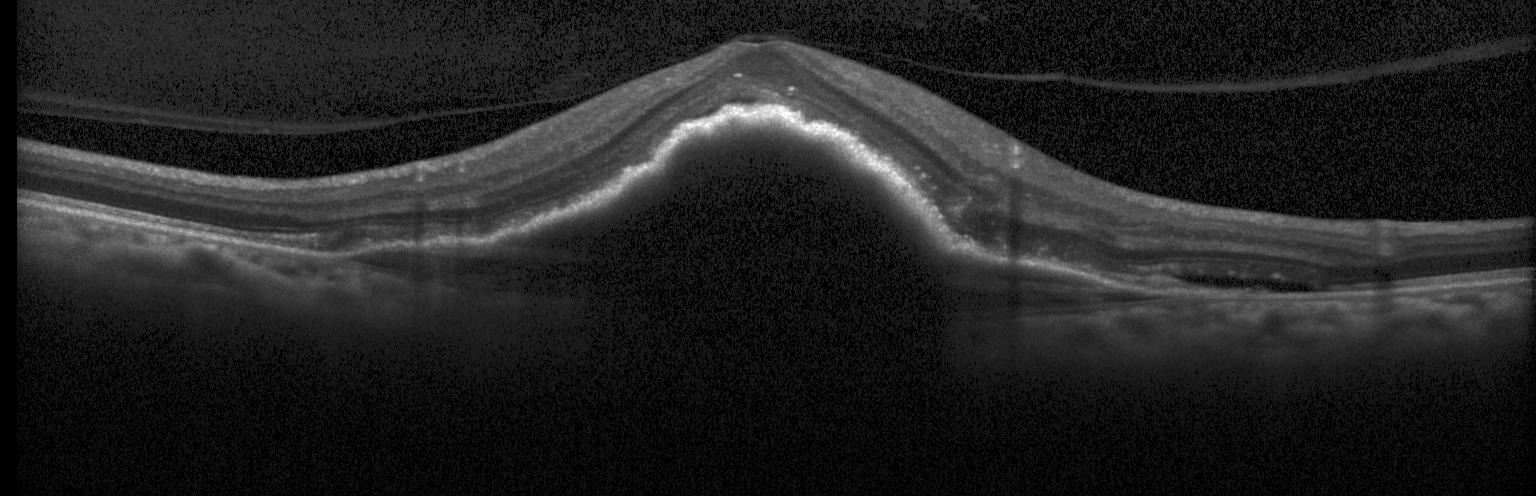
Heidelberg Spectralis, OCT B-scan.
Finding: a choroidal neovascular membrane.